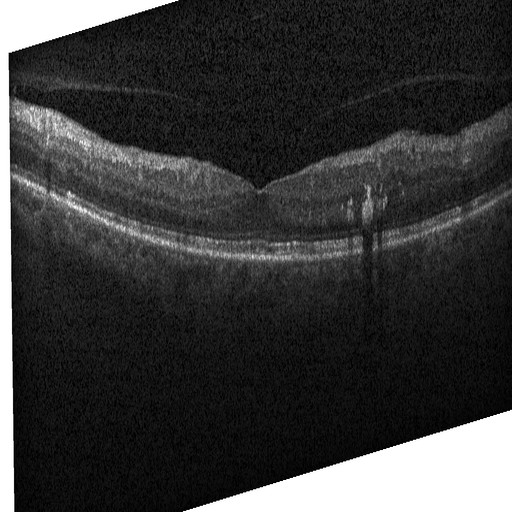
Finding: diabetic macular edema.